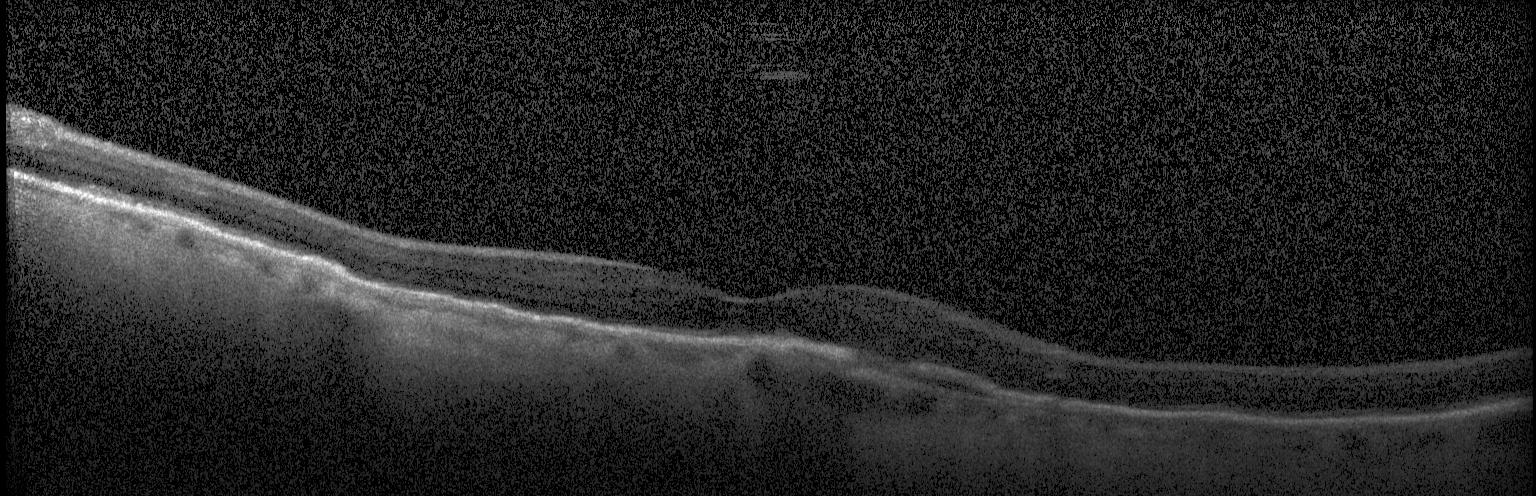

Macular scan, OCT B-scan, Heidelberg Spectralis OCT system, spectral-domain optical coherence tomography
Impression: choroidal neovascularization.